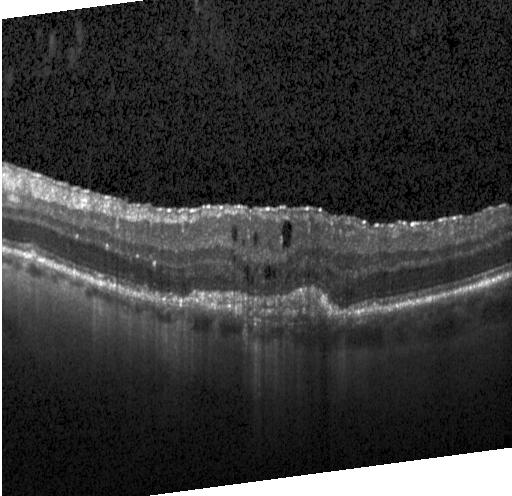
OCT B-scan; Heidelberg Spectralis; through the macula; SD-OCT. The scan shows a choroidal neovascular membrane.